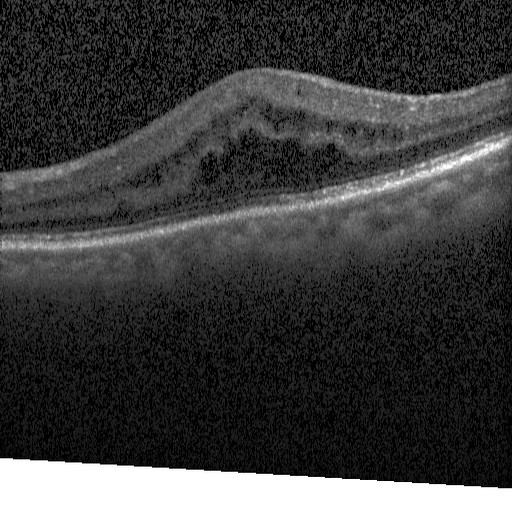

OCT scan showing diabetic macular edema (DME).